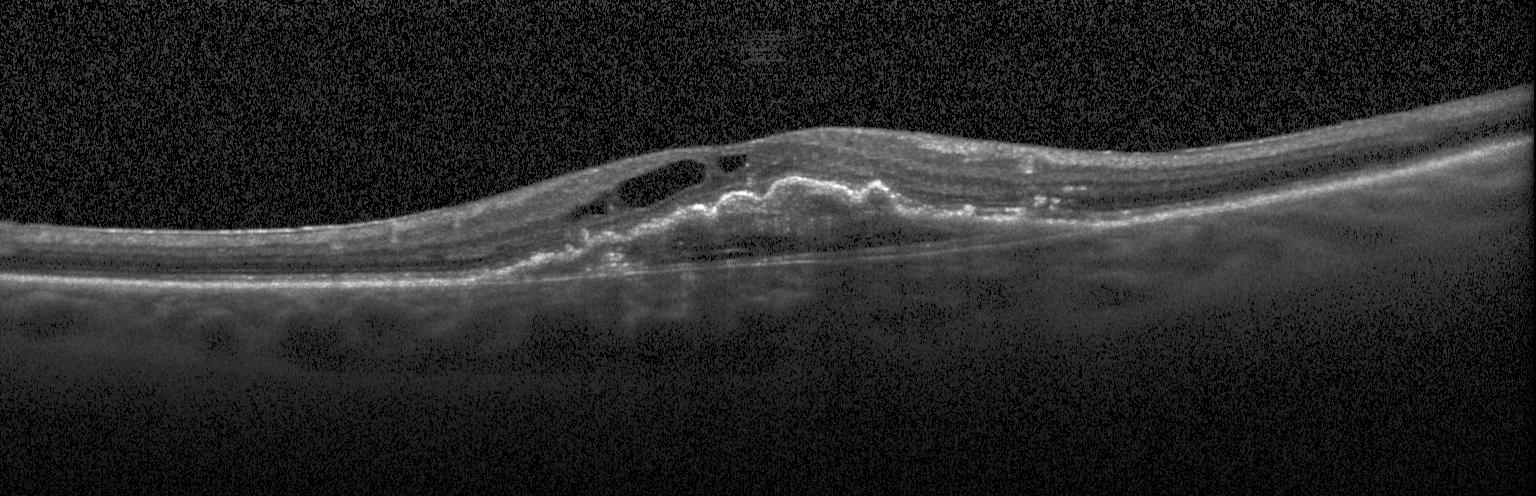
Retinal OCT cross-section · acquired on a Heidelberg Spectralis · spectral-domain optical coherence tomography — OCT finding: a choroidal neovascular membrane.